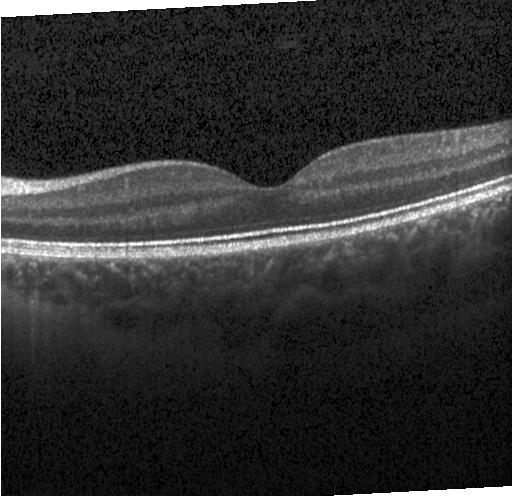 Macular OCT: no evidence of choroidal neovascularization, diabetic macular edema, or drusen.